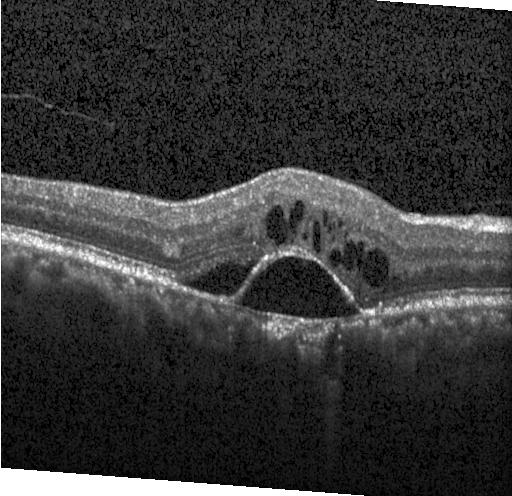

Optical coherence tomography scan. Fovea-centered. Heidelberg Spectralis. Spectral-domain OCT — This B-scan demonstrates a choroidal neovascular membrane.